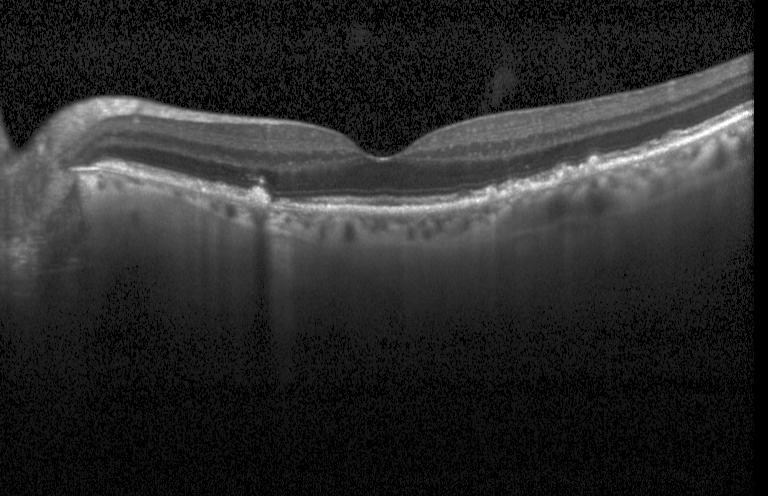
Assessment: sub-RPE drusenoid deposits.